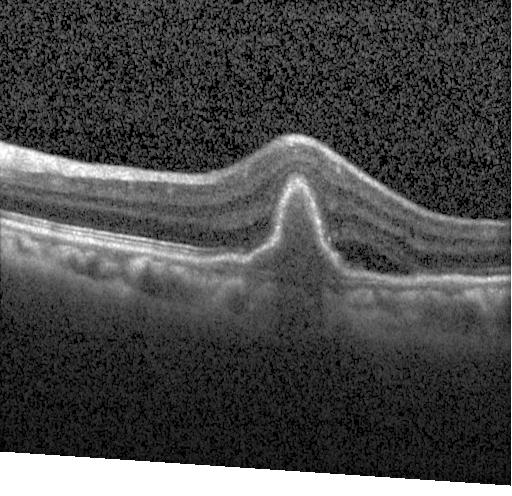
This B-scan demonstrates choroidal neovascularization (CNV).